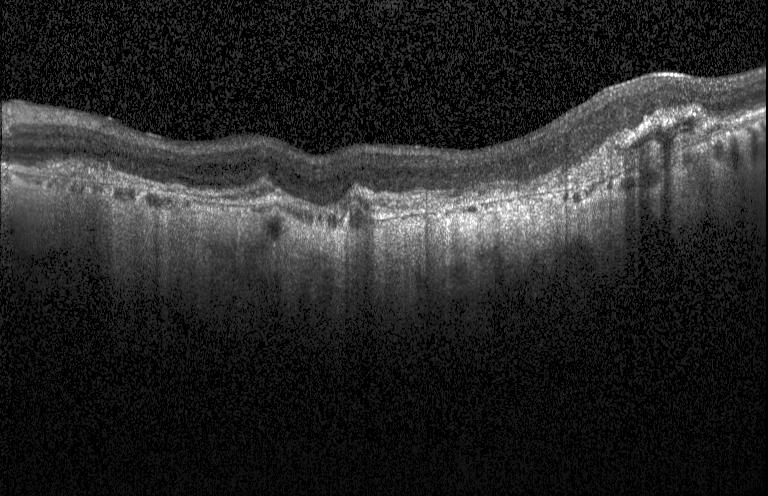

Impression: CNV.